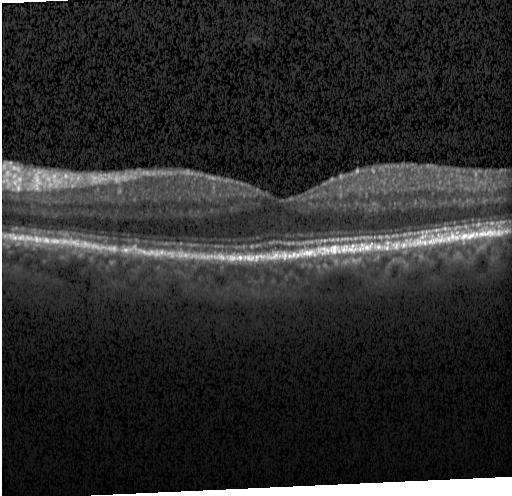

Impression: neither choroidal neovascularization, diabetic macular edema, nor drusen.